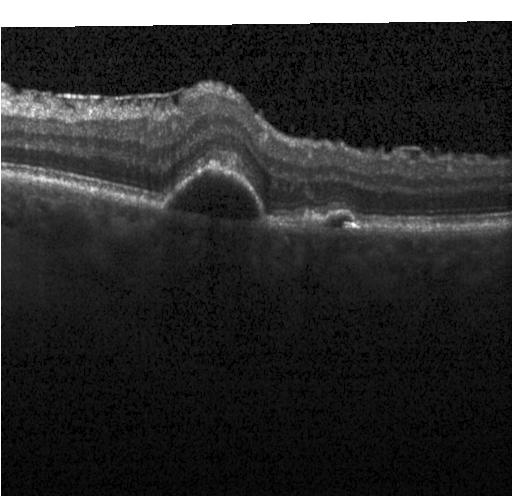 Optical coherence tomography B-scan
Finding: a choroidal neovascular membrane.